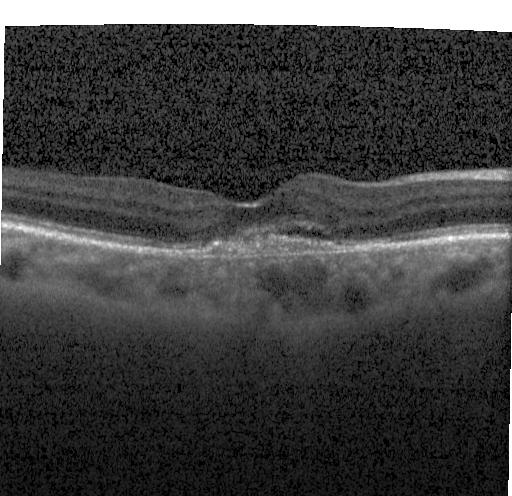
Retinal OCT cross-section · centered on the fovea.
Finding: choroidal neovascularization.